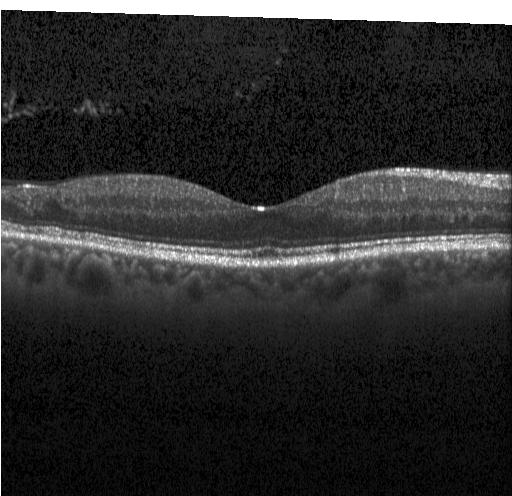 Heidelberg Spectralis; horizontal scan through the fovea; optical coherence tomography scan; spectral-domain optical coherence tomography
Assessment: neither CNV, DME, nor drusen.